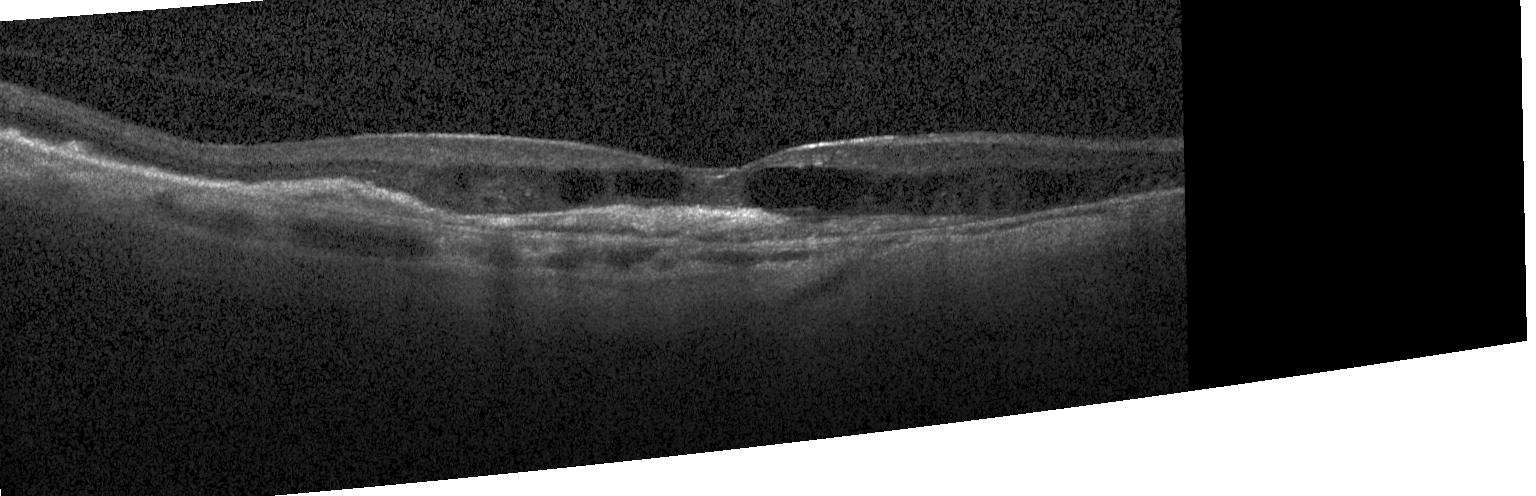

Retinal OCT cross-section; spectral-domain optical coherence tomography. Diagnosis: a choroidal neovascular membrane.